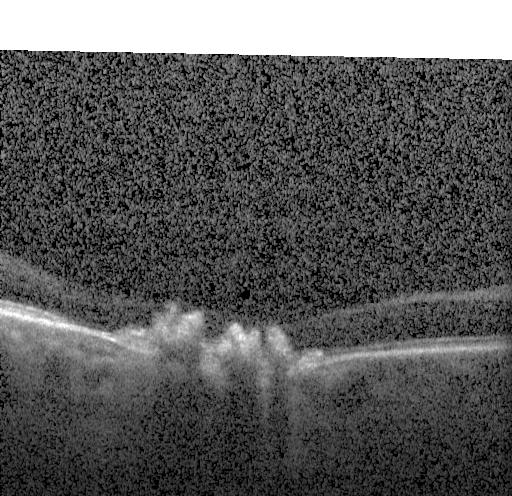
Macular OCT: CNV.